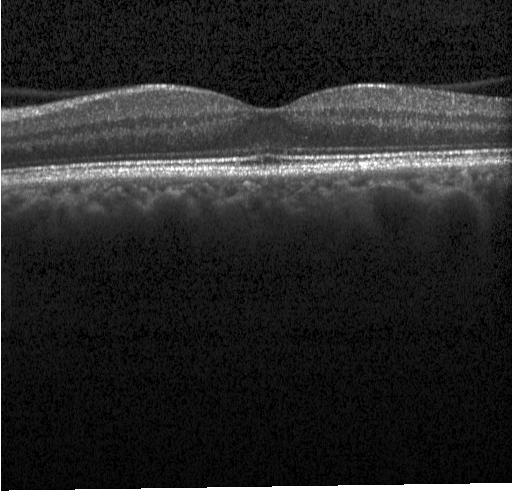

Spectral-domain optical coherence tomography, retinal OCT B-scan
No evidence of CNV, DME, or drusen.